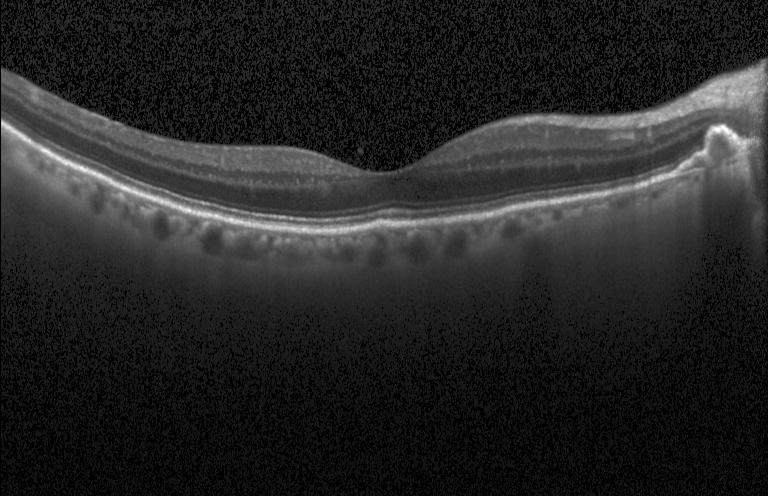 Optical coherence tomography scan, acquired on a Heidelberg Spectralis
A choroidal neovascular membrane.